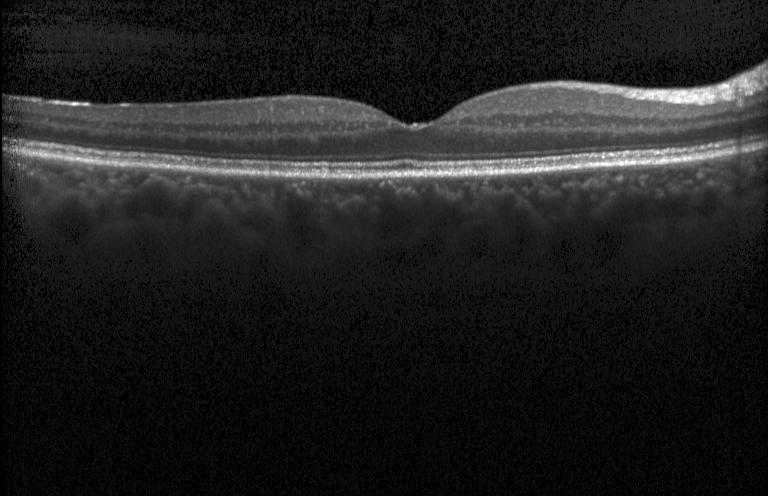 OCT finding: no evidence of choroidal neovascularization, diabetic macular edema, or drusen.